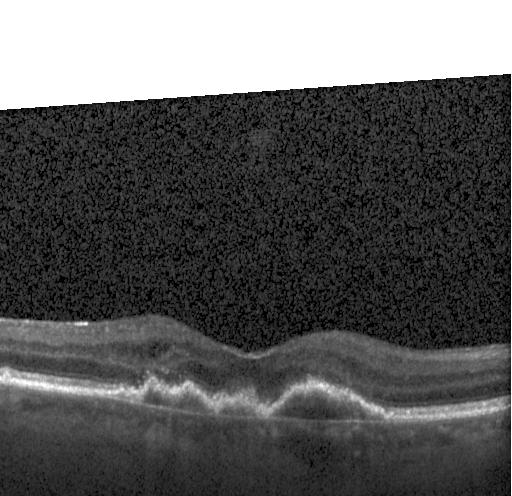

Diagnosis: a choroidal neovascular membrane.